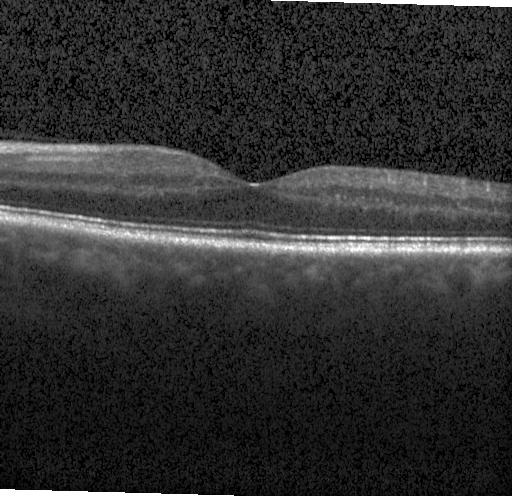

OCT B-scan, SD-OCT, macular scan, Heidelberg Spectralis
Diagnosis: neither CNV, DME, nor drusen.